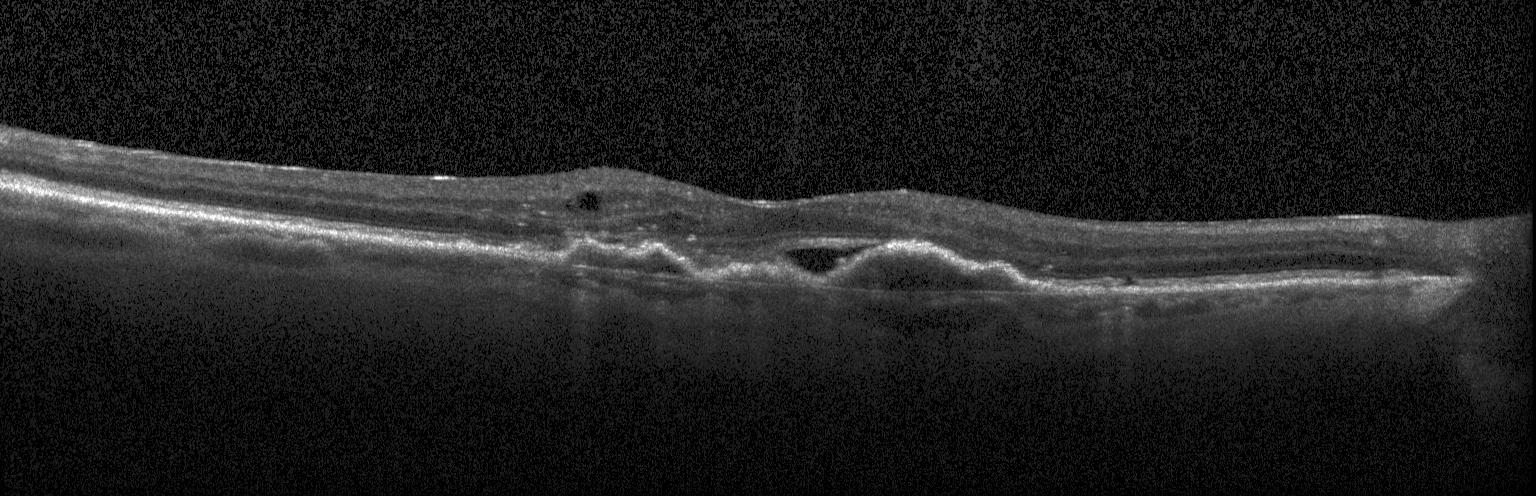 Impression: a choroidal neovascular membrane.